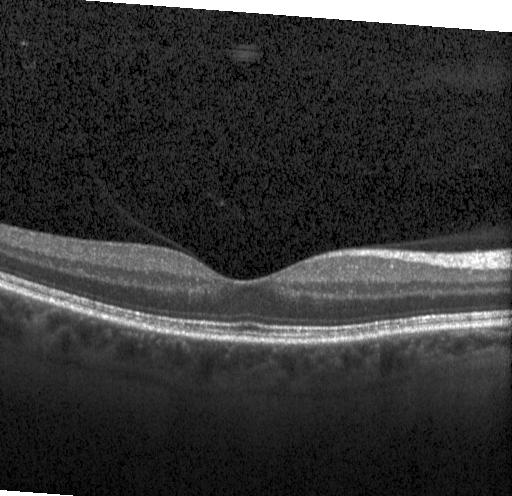

Retinal OCT B-scan · fovea-centered · acquired on a Heidelberg Spectralis. No choroidal neovascularization, diabetic macular edema, or drusen.